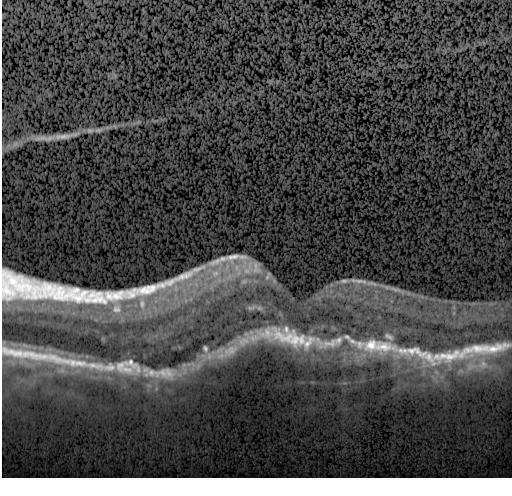 Retinal OCT cross-section, SD-OCT, fovea-centered. Assessment: choroidal neovascularization (CNV).